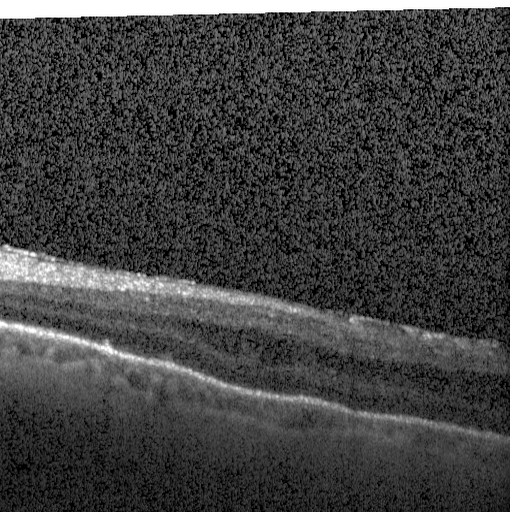
Impression: diabetic macular edema.